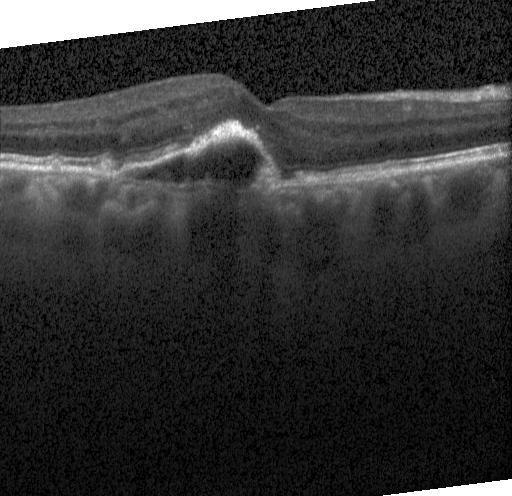
Impression: a choroidal neovascular membrane.